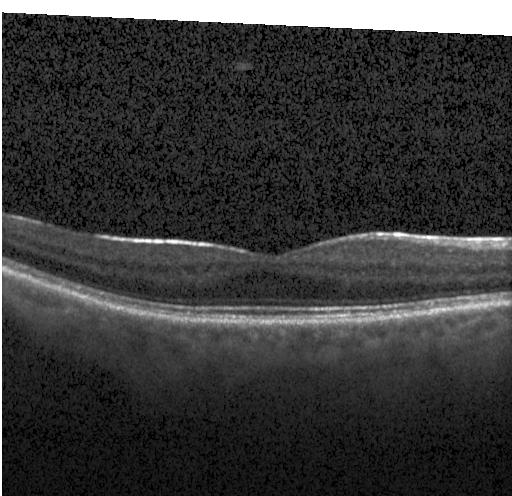
Spectral-domain OCT B-scan: no CNV, DME, or drusen.